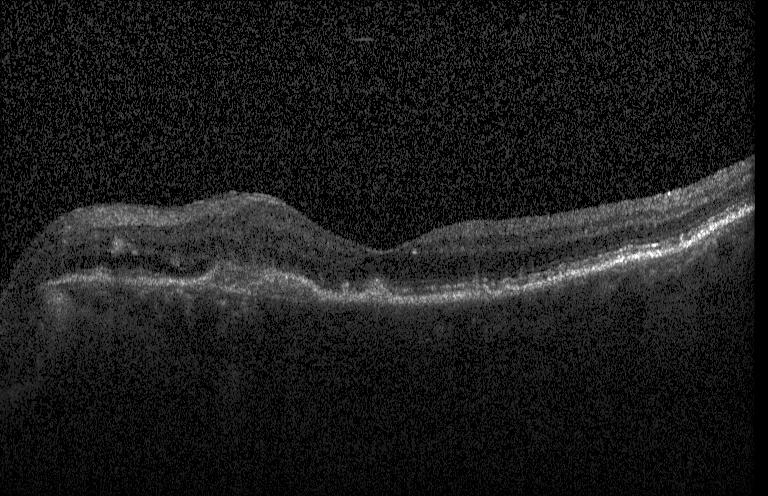
Instrument: Heidelberg Spectralis, optical coherence tomography B-scan, through the macula. Finding: choroidal neovascularization.